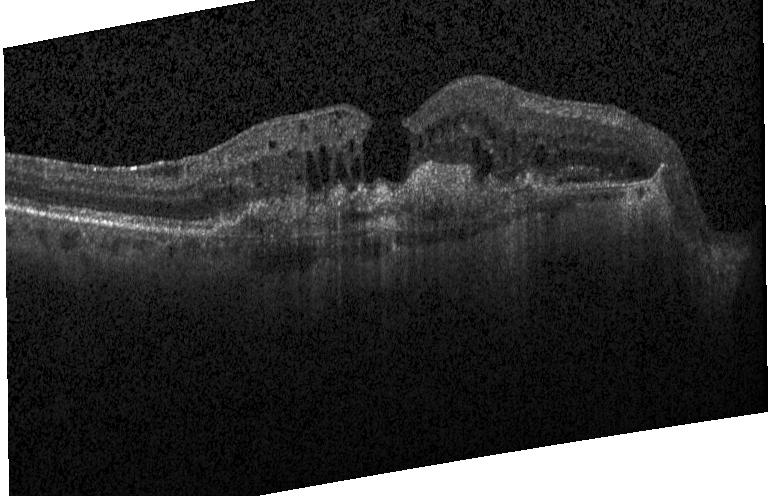 Heidelberg Spectralis. OCT B-scan. Centered on the fovea — Assessment: choroidal neovascularization.